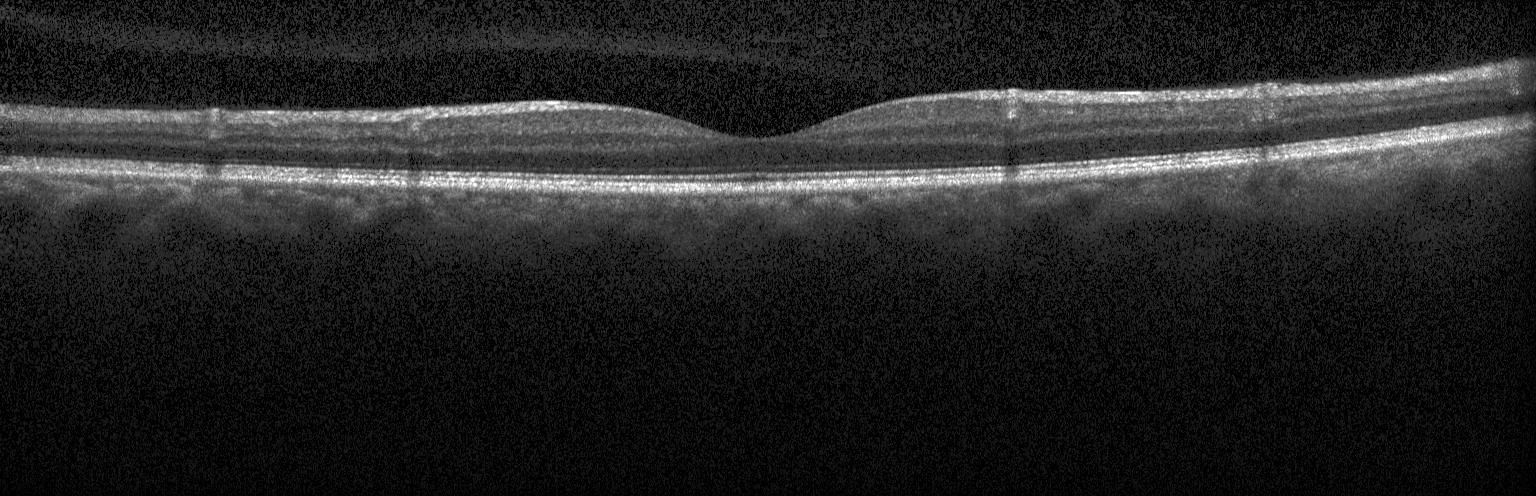

Optical coherence tomography B-scan, spectral-domain optical coherence tomography
Finding: no evidence of choroidal neovascularization, diabetic macular edema, or drusen.